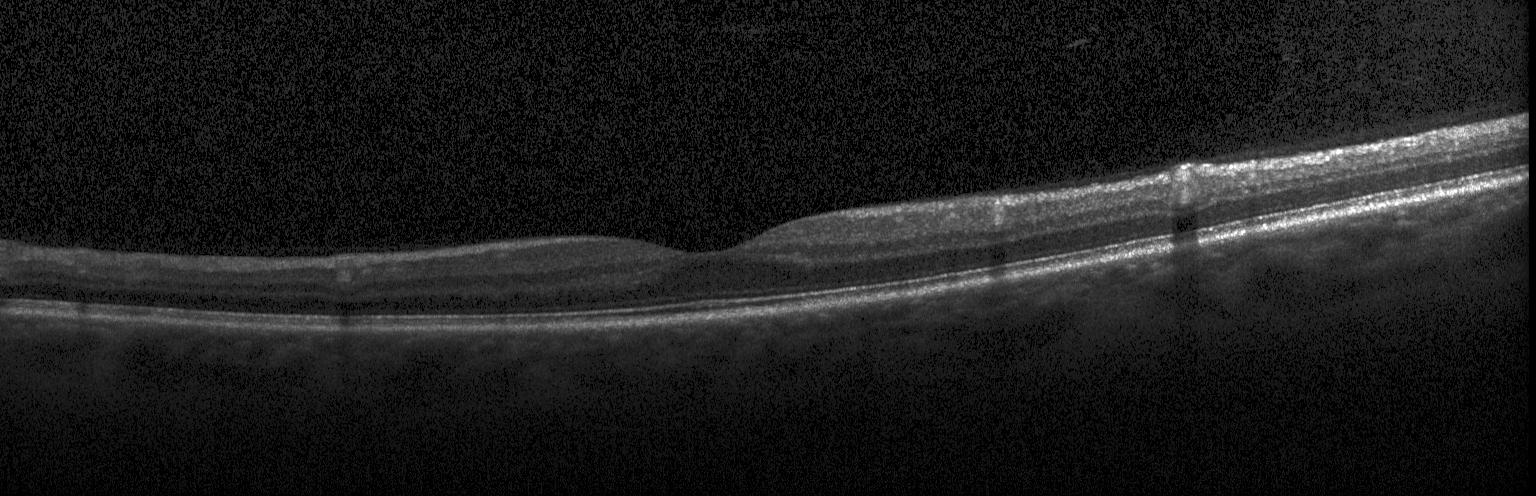
Spectral-domain optical coherence tomography · retinal OCT cross-section. This B-scan demonstrates no evidence of choroidal neovascularization, diabetic macular edema, or drusen.